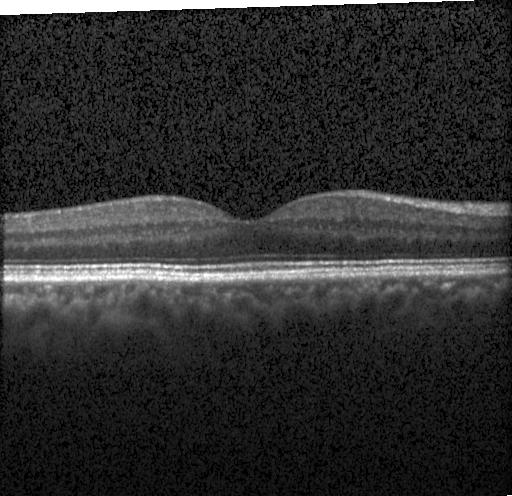
This B-scan demonstrates no evidence of choroidal neovascularization, diabetic macular edema, or drusen.